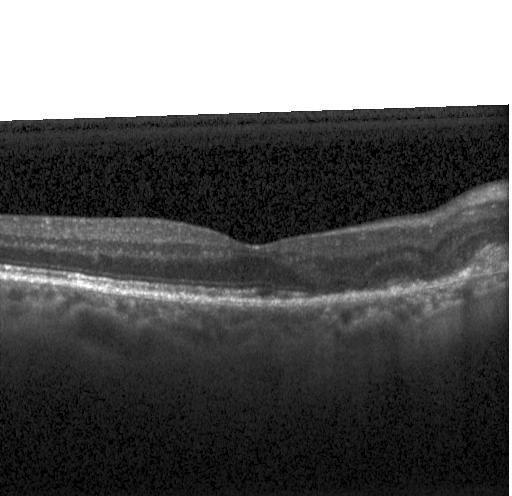 Diagnosis: choroidal neovascularization (CNV).